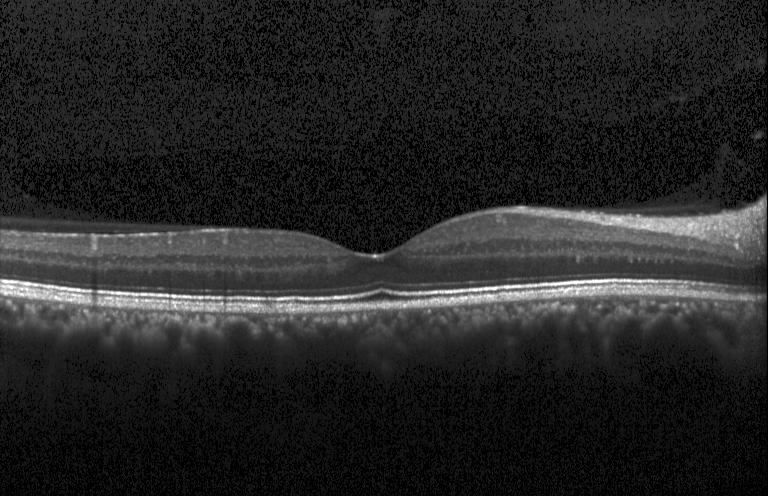 No choroidal neovascularization, no diabetic macular edema, and no drusen.